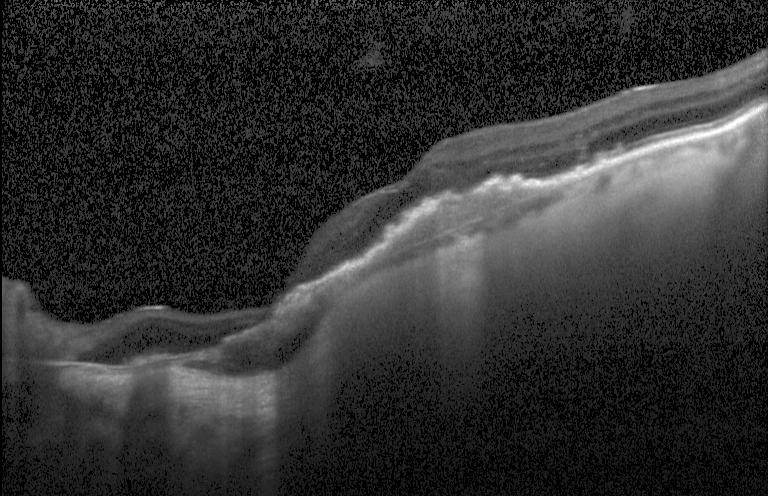
Spectral-domain optical coherence tomography; centered on the fovea; retinal OCT cross-section
Finding: choroidal neovascularization (CNV).